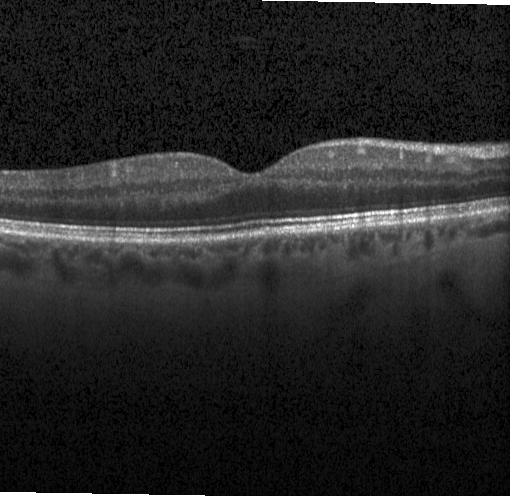
Finding: no choroidal neovascularization, no diabetic macular edema, and no drusen.